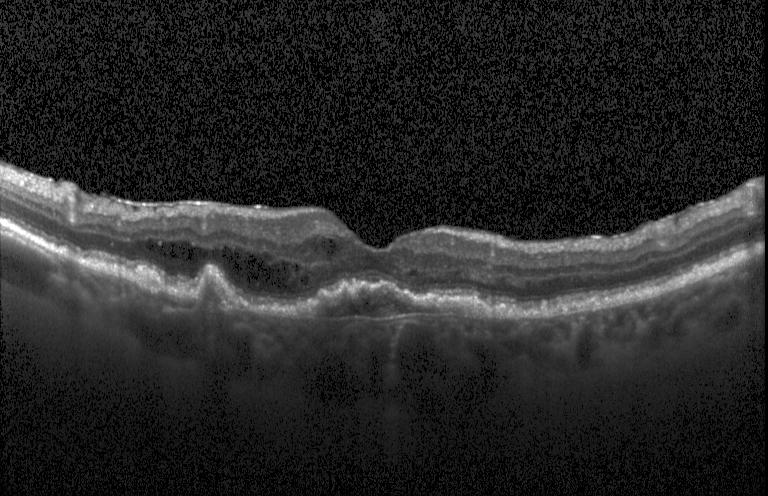
OCT B-scan. The scan shows a choroidal neovascular membrane.